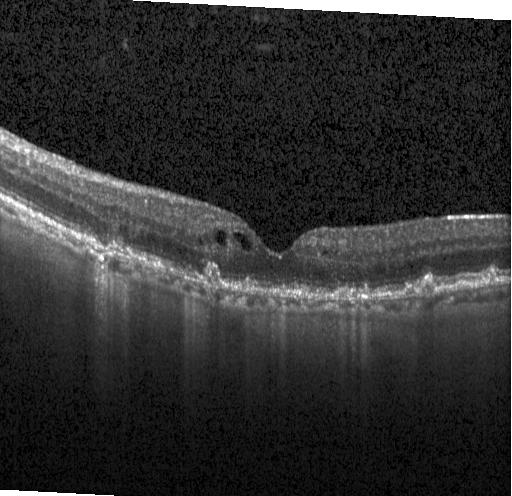
Optical coherence tomography scan; acquired on a Heidelberg Spectralis; horizontal scan through the fovea. Finding: CNV.